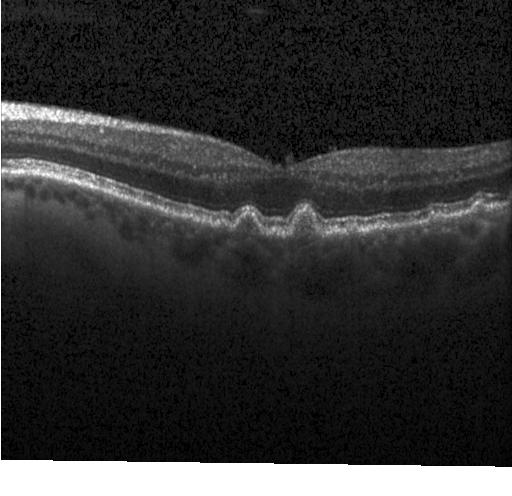 Optical coherence tomography B-scan
OCT finding: sub-RPE drusenoid deposits.